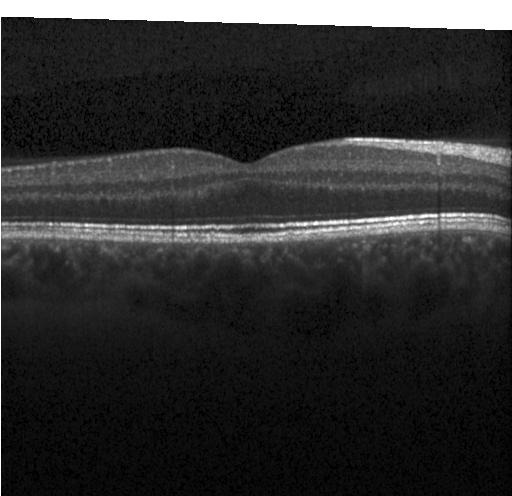

Horizontal scan through the fovea; spectral-domain optical coherence tomography; retinal OCT cross-section
Neither choroidal neovascularization, diabetic macular edema, nor drusen.